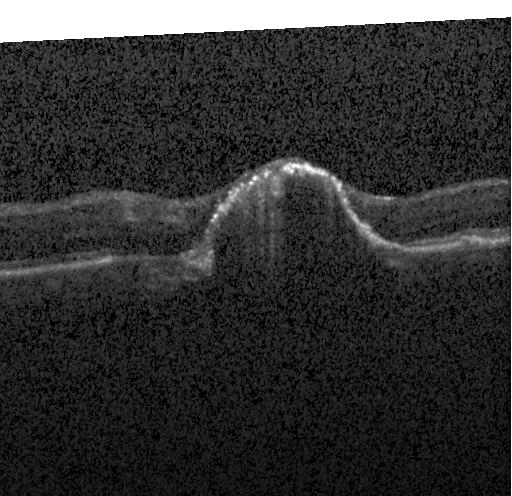

Heidelberg Spectralis OCT system · retinal OCT cross-section · macular scan — Diagnosis: choroidal neovascularization.